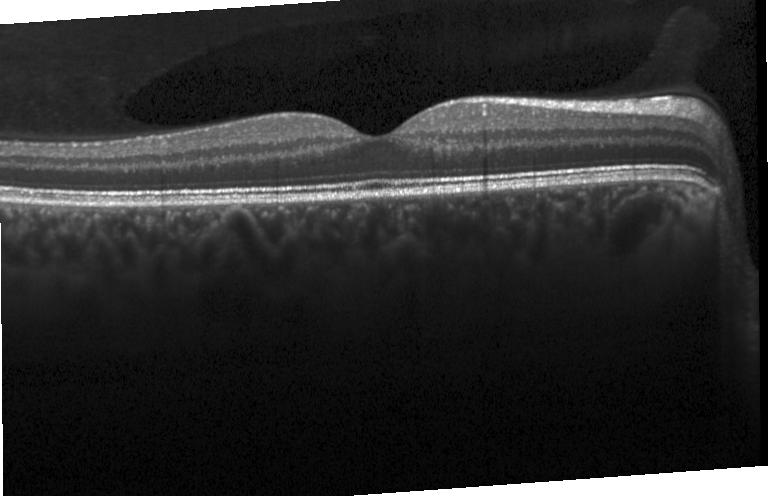
Optical coherence tomography scan. Through the macula. Spectral-domain OCT.
Neither choroidal neovascularization, diabetic macular edema, nor drusen.